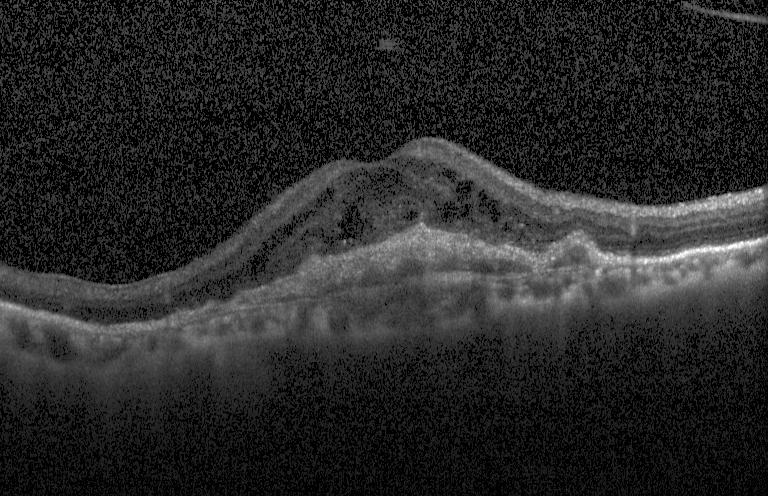
Retinal OCT B-scan. OCT finding: a choroidal neovascular membrane.